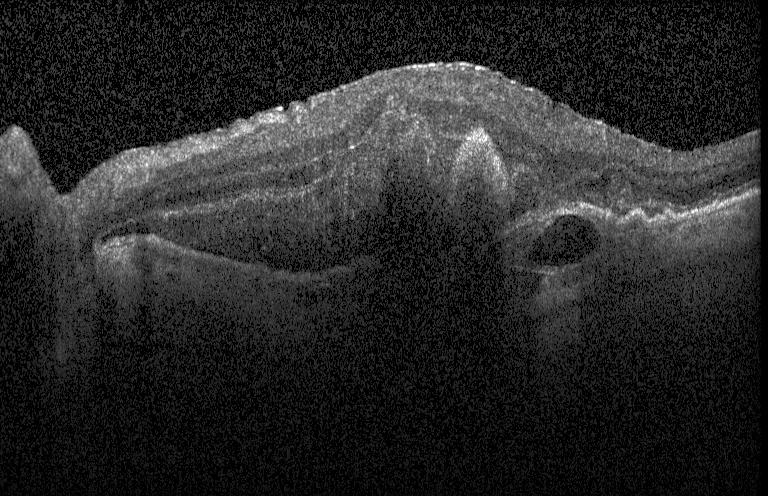
Fovea-centered · SD-OCT · Heidelberg Spectralis · retinal OCT cross-section — OCT finding: CNV.